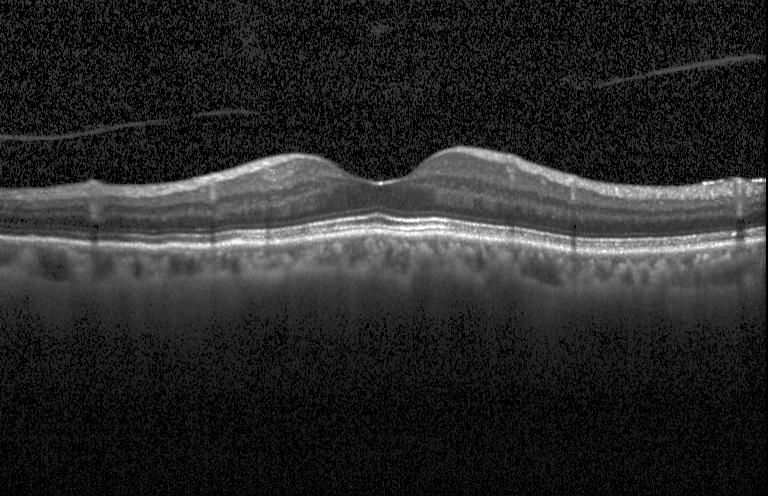

Spectral-domain OCT B-scan: no choroidal neovascularization, diabetic macular edema, or drusen.